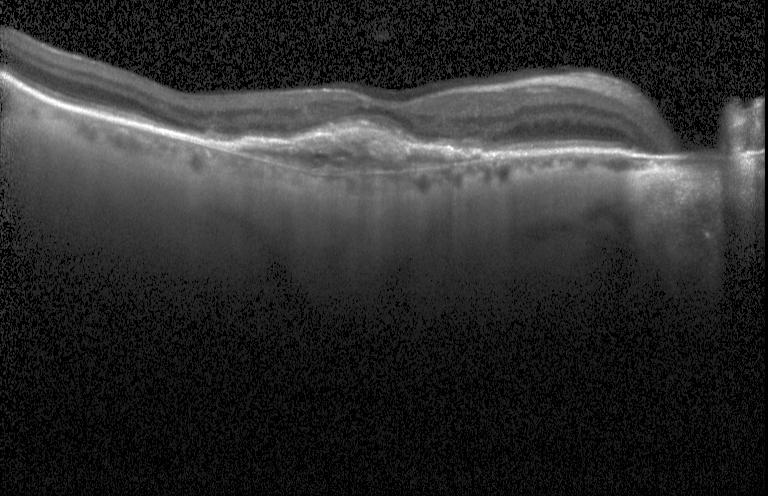 Optical coherence tomography B-scan. Spectral-domain optical coherence tomography. Heidelberg Spectralis OCT system.
Assessment: a choroidal neovascular membrane.